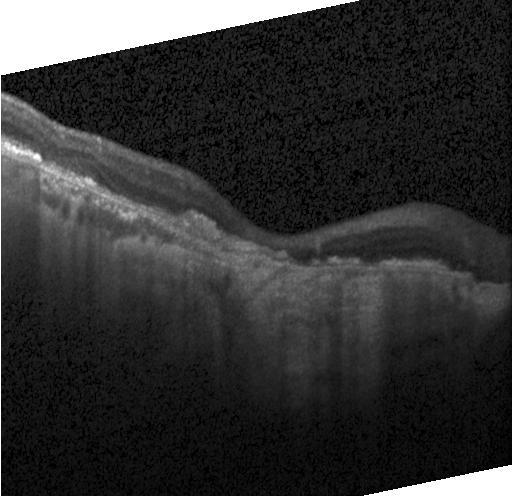
Retinal OCT B-scan · Heidelberg Spectralis OCT system · fovea-centered · spectral-domain optical coherence tomography
Assessment: a choroidal neovascular membrane.